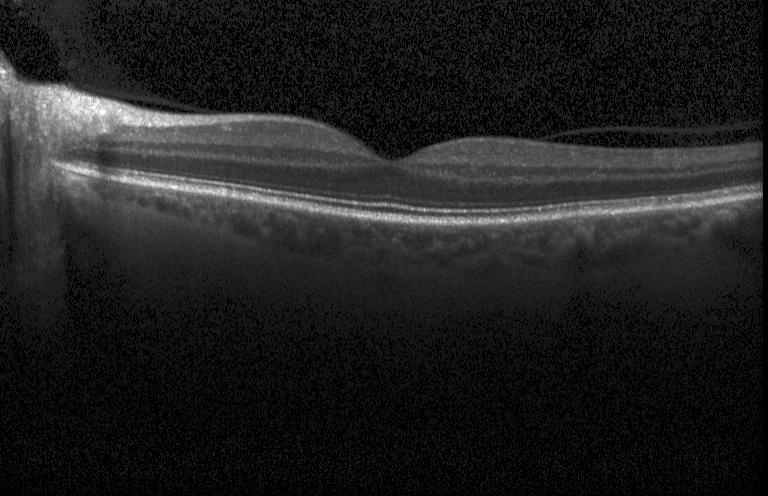
Impression: neither choroidal neovascularization, diabetic macular edema, nor drusen.